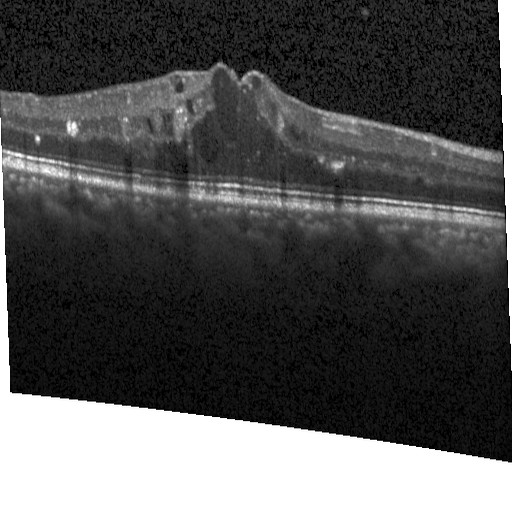

Optical coherence tomography scan · spectral-domain OCT · macular scan — Macular OCT: diabetic macular edema.